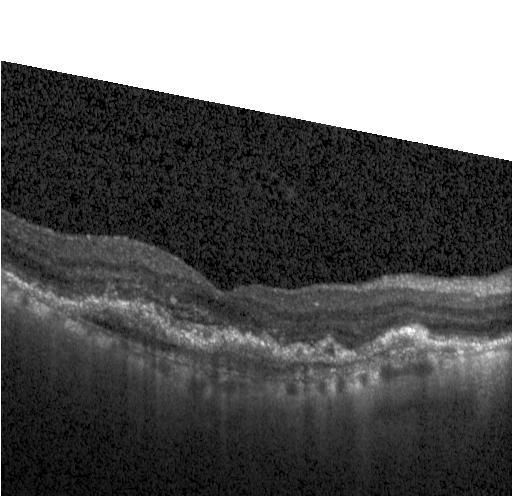
Retinal OCT cross-section showing a choroidal neovascular membrane.